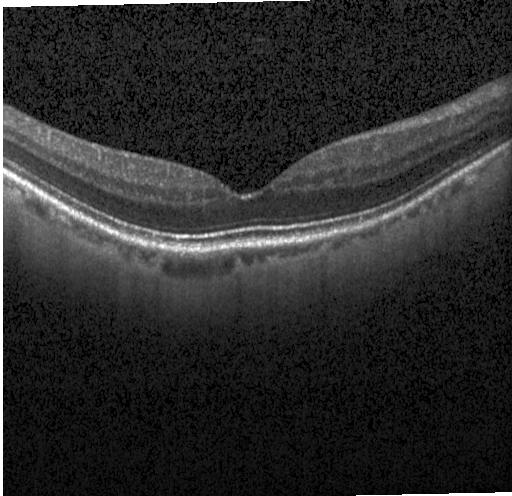
Diagnosis: no evidence of choroidal neovascularization, diabetic macular edema, or drusen.